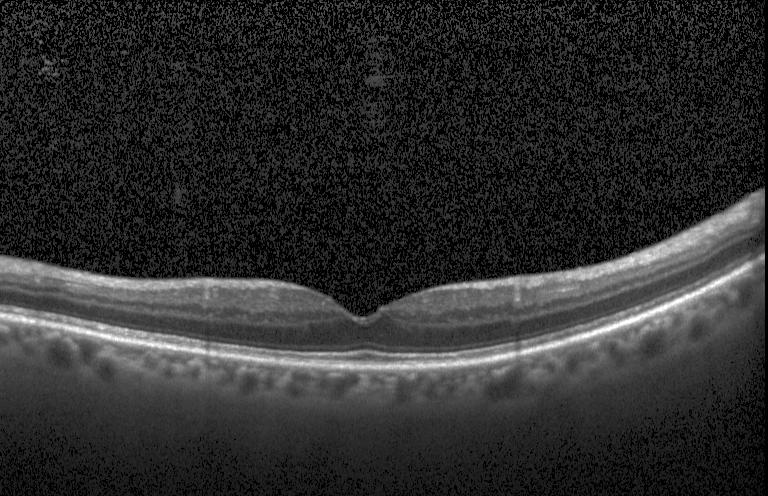
The scan shows no evidence of CNV, DME, or drusen.